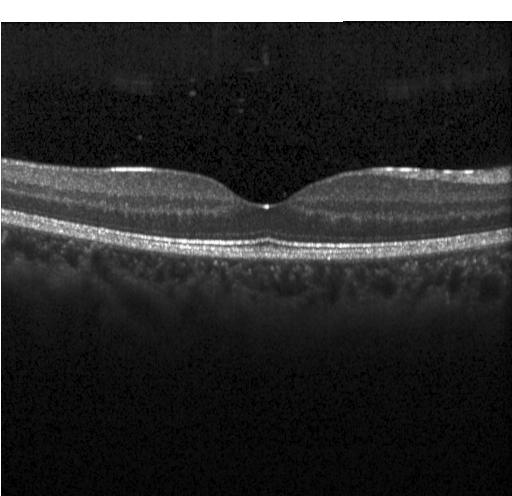

Finding: no evidence of choroidal neovascularization, diabetic macular edema, or drusen.